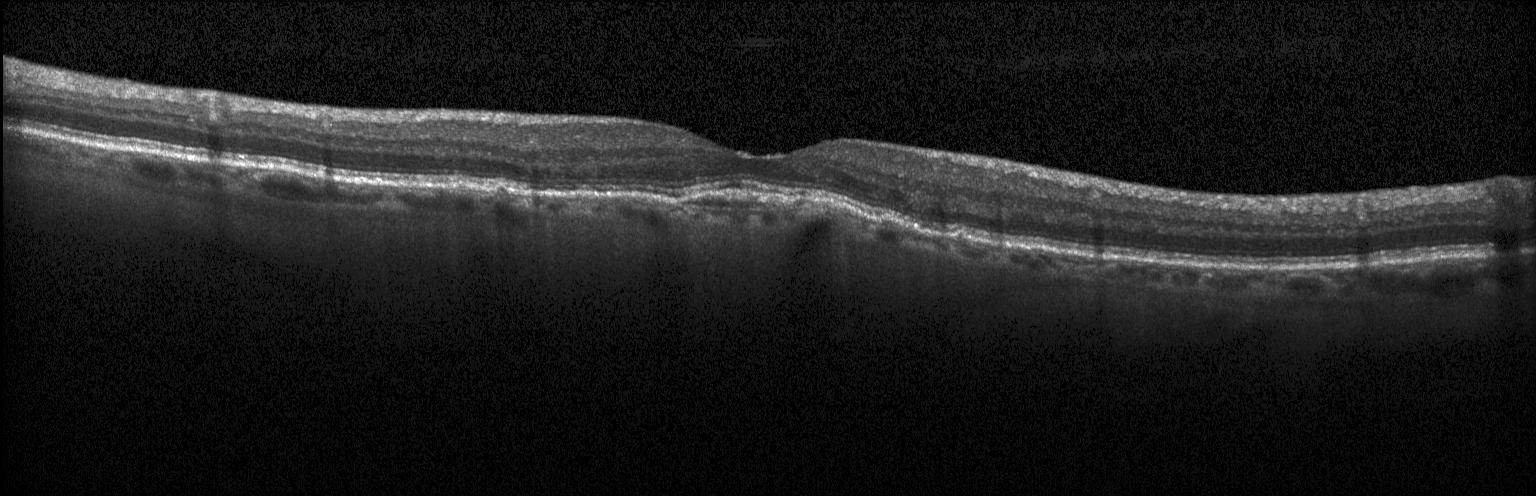

Diagnosis: choroidal neovascularization (CNV).